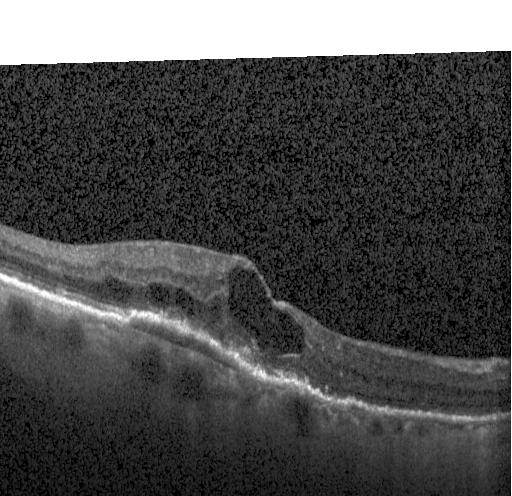

Optical coherence tomography B-scan · fovea-centered. The scan shows choroidal neovascularization (CNV).